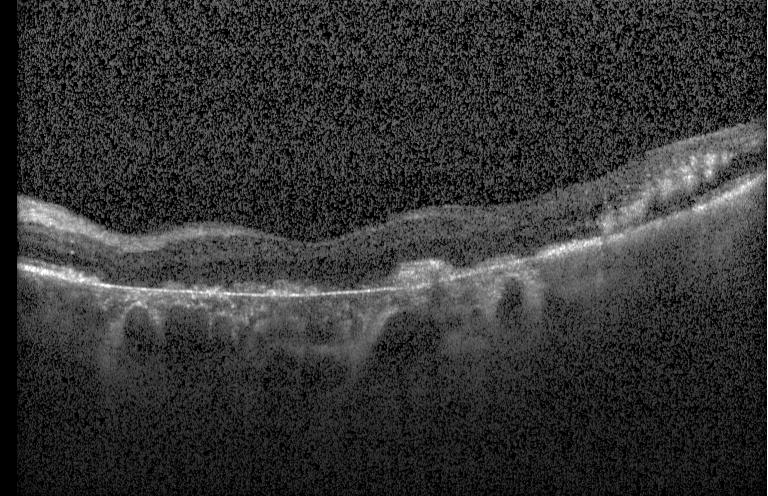
Fovea-centered. Heidelberg Spectralis OCT system. OCT B-scan. Spectral-domain optical coherence tomography — A choroidal neovascular membrane.